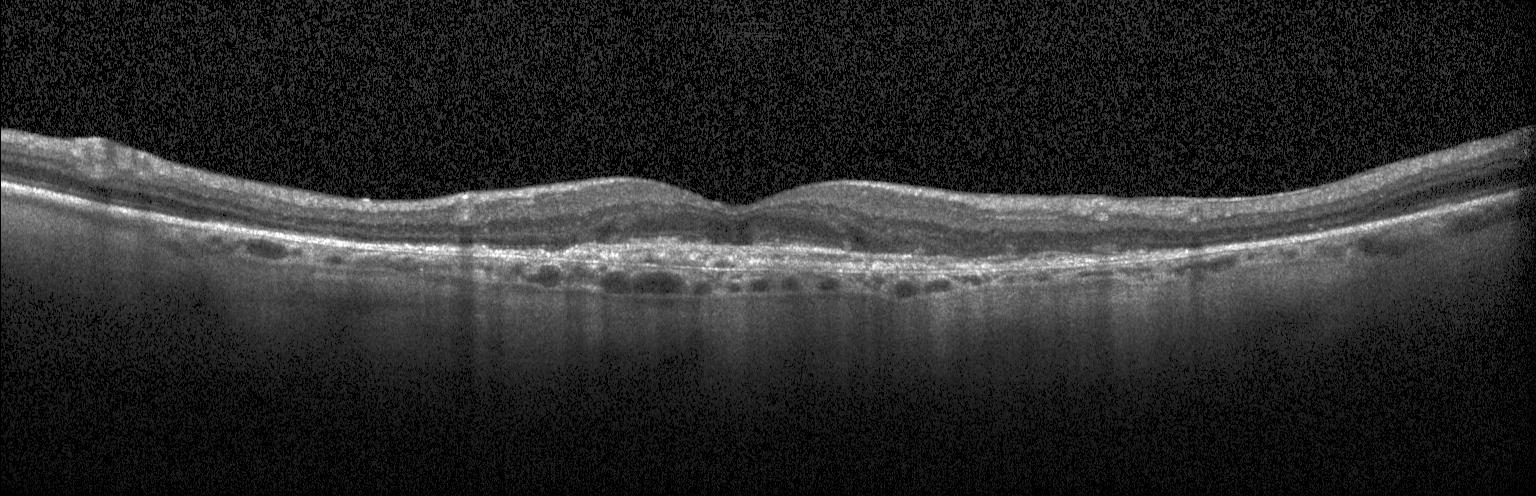 The scan shows choroidal neovascularization (CNV).